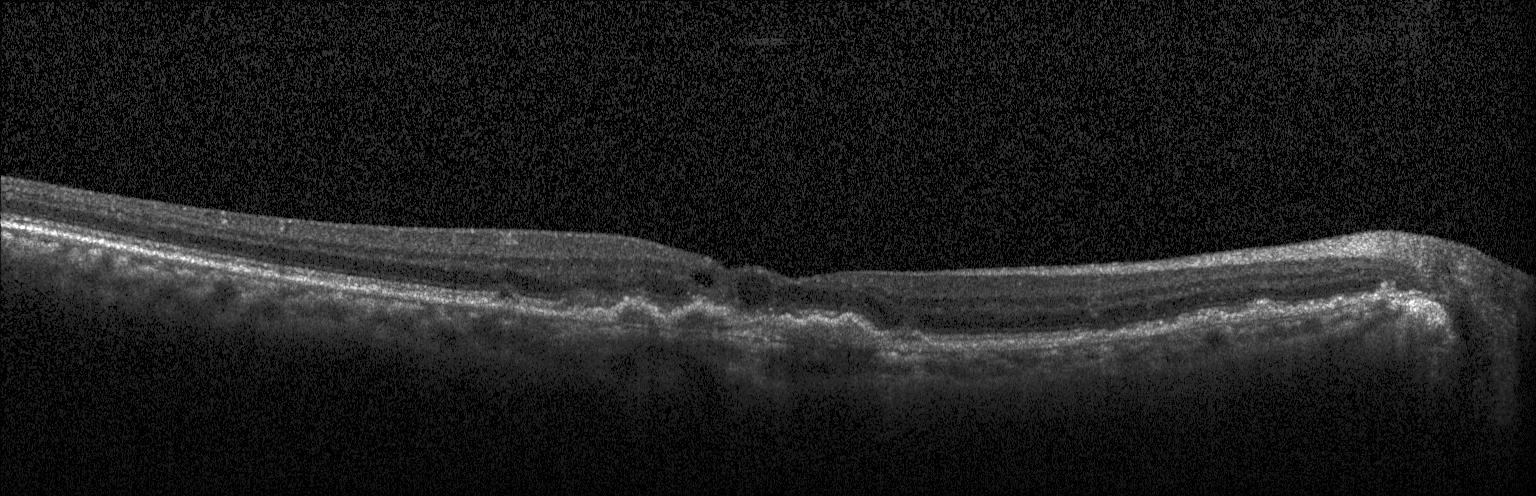 Spectral-domain OCT B-scan: a choroidal neovascular membrane.